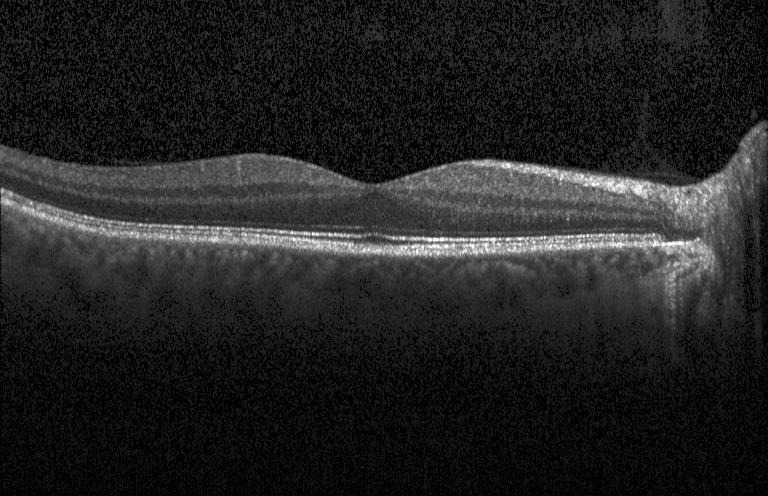

Optical coherence tomography scan, centered on the fovea.
Dx: neither choroidal neovascularization, diabetic macular edema, nor drusen.